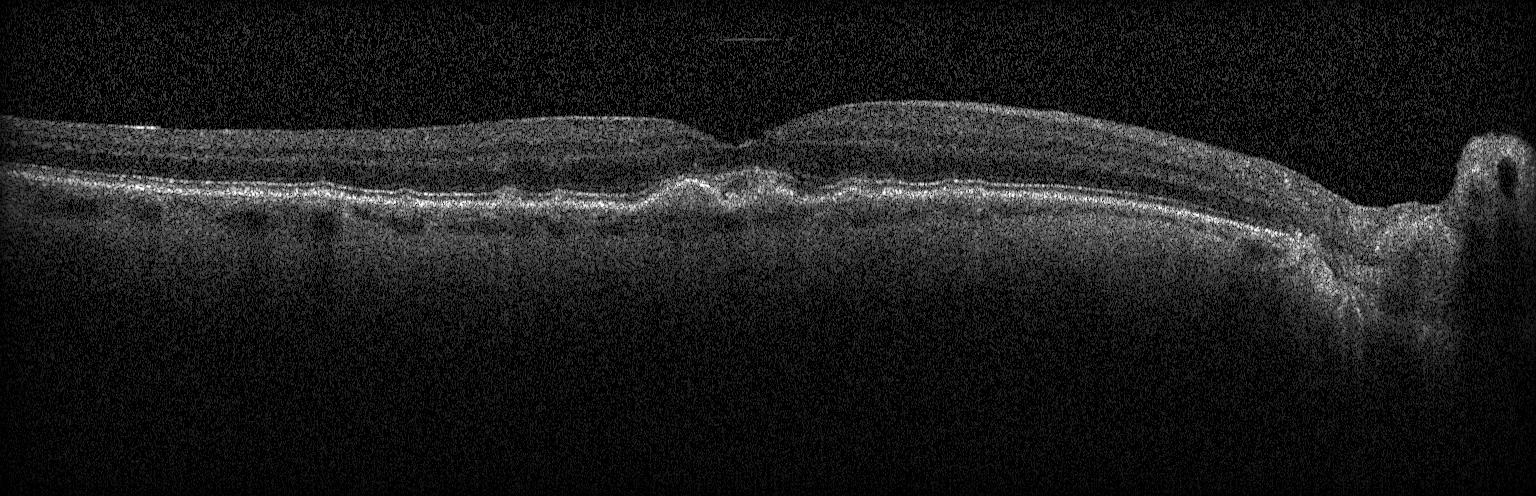

Dx: multiple drusen.